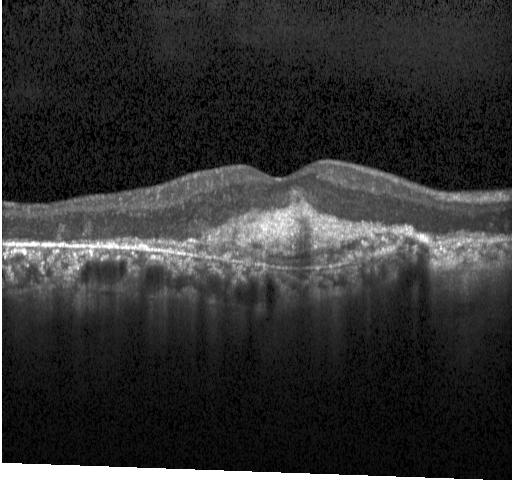

Heidelberg Spectralis. Optical coherence tomography B-scan. Centered on the fovea.
Diagnosis: a choroidal neovascular membrane.